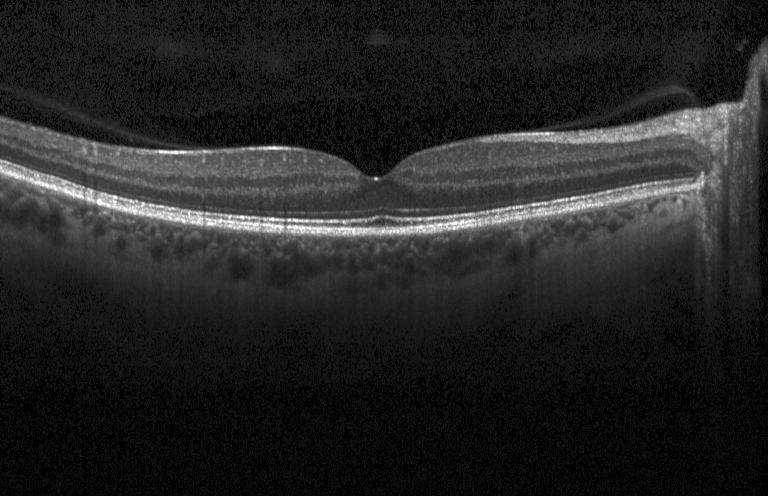
Optical coherence tomography B-scan, SD-OCT, Heidelberg Spectralis OCT system, through the macula — This B-scan demonstrates no choroidal neovascularization, no diabetic macular edema, and no drusen.